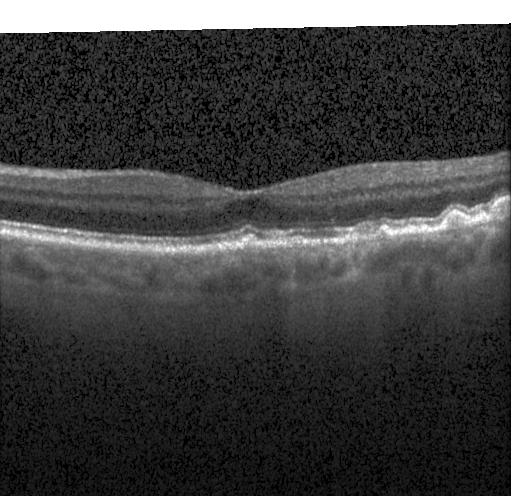 Retinal OCT cross-section · macular scan · spectral-domain OCT — Finding: drusen.